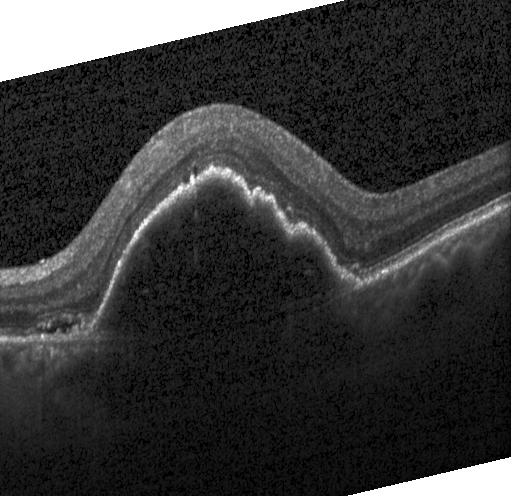

Diagnosis: a choroidal neovascular membrane.